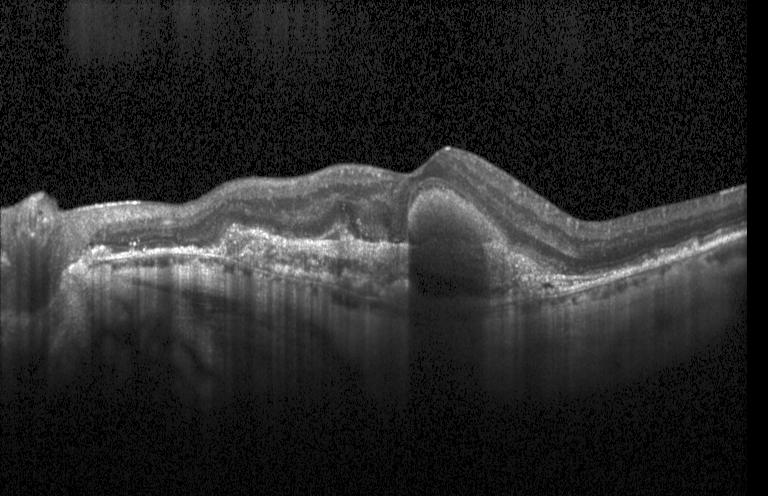

The scan shows choroidal neovascularization (CNV).